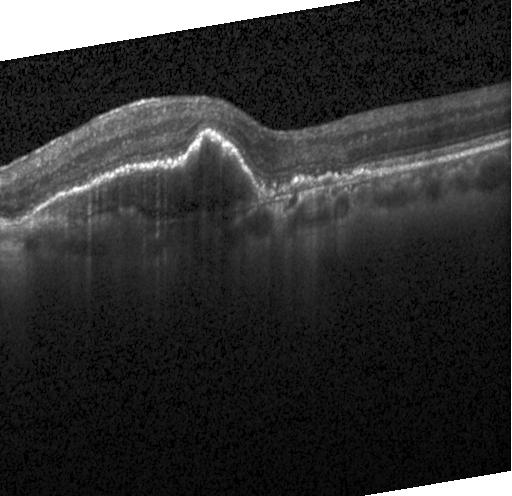

Optical coherence tomography scan
Finding: choroidal neovascularization (CNV).